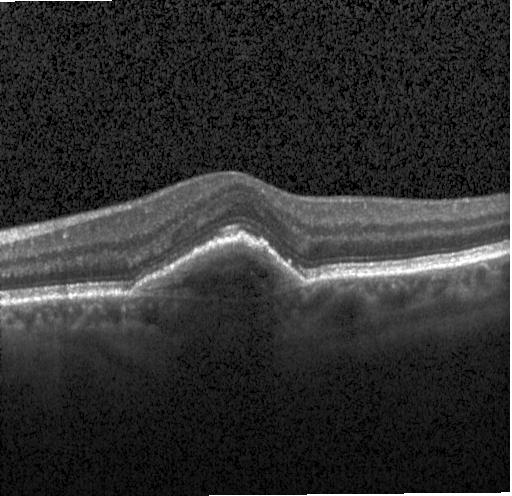 Impression: a choroidal neovascular membrane.